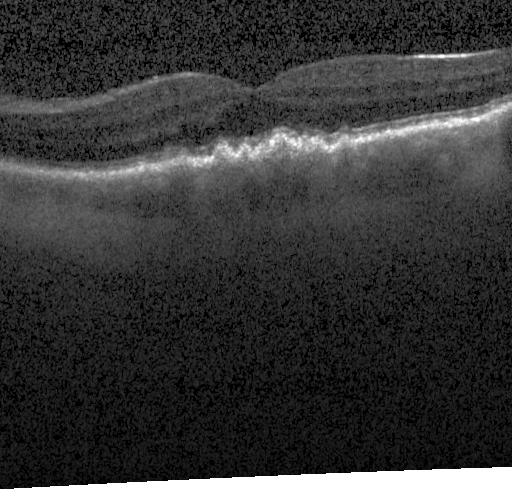 Dx: sub-RPE drusenoid deposits.